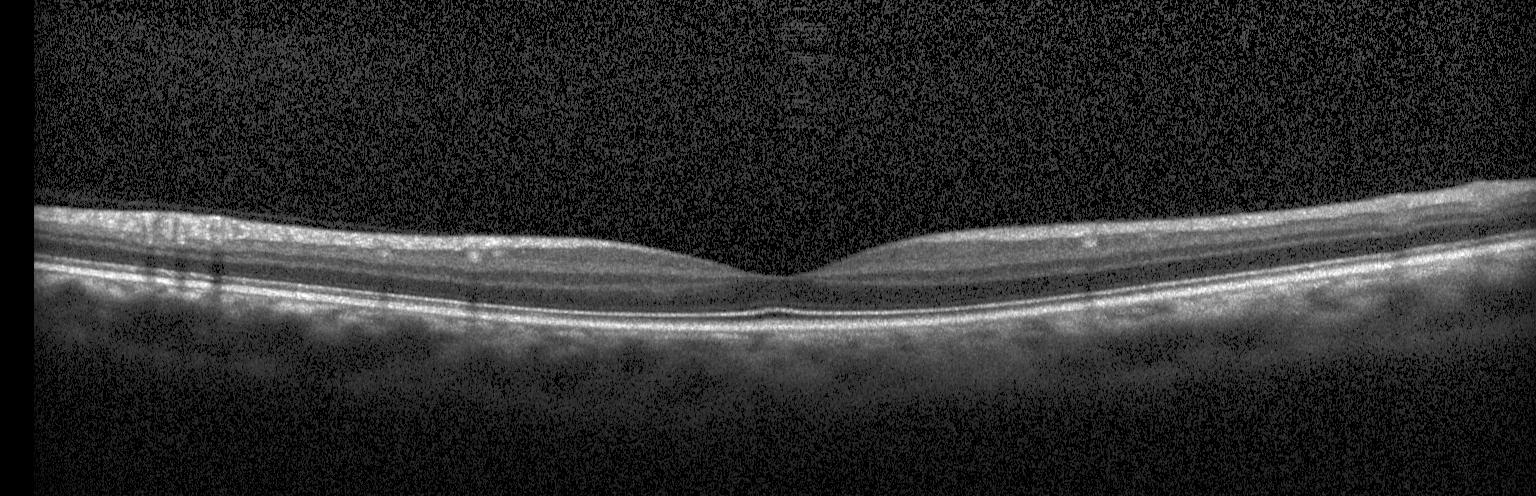
The scan shows neither CNV, DME, nor drusen.